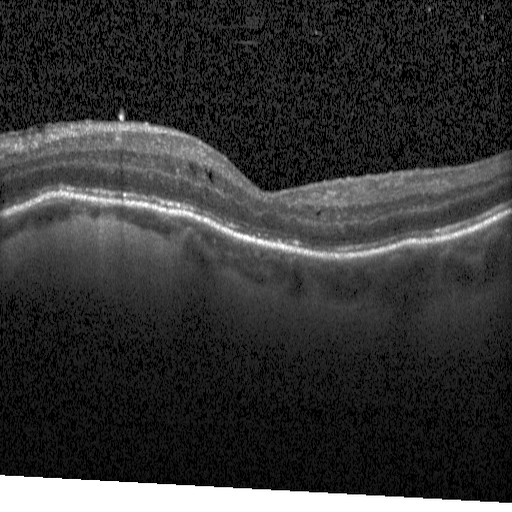 Through the macula · retinal OCT cross-section · spectral-domain optical coherence tomography · instrument: Heidelberg Spectralis
The scan shows DME.